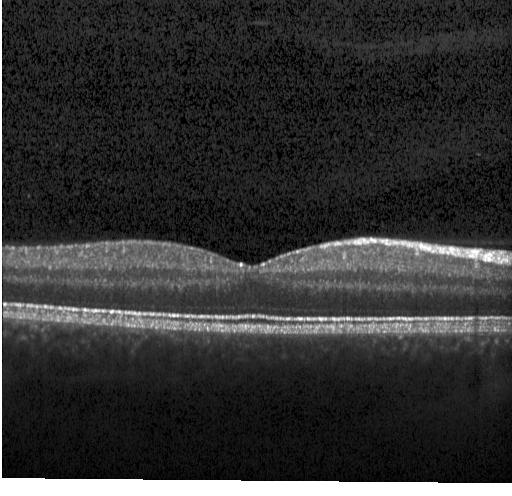

OCT line scan. This B-scan demonstrates no choroidal neovascularization, no diabetic macular edema, and no drusen.